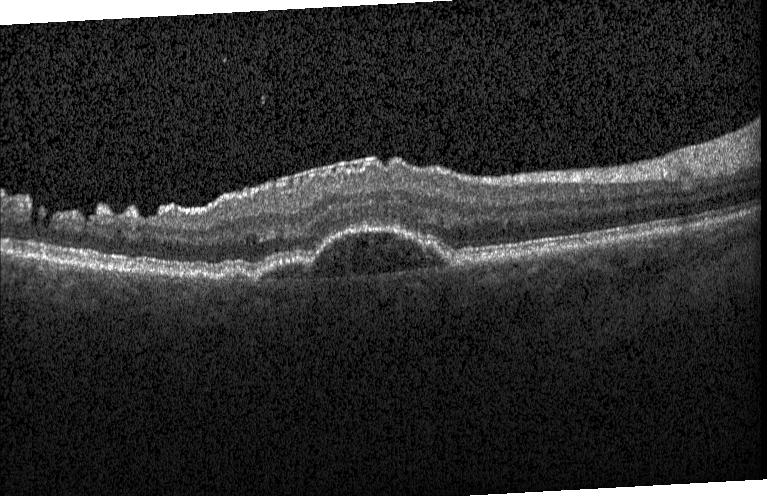
Optical coherence tomography B-scan · centered on the fovea · acquired on a Heidelberg Spectralis
Diagnosis: choroidal neovascularization (CNV).